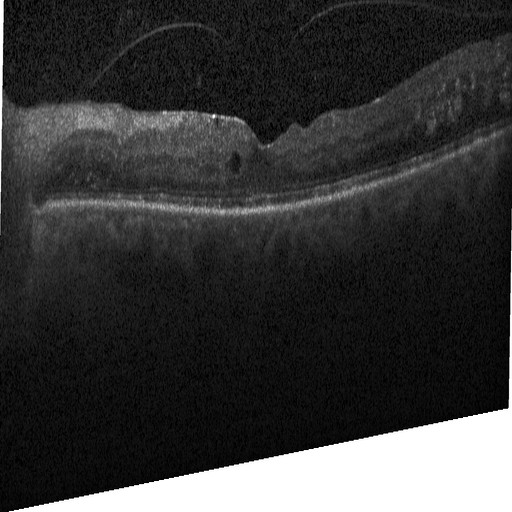 OCT scan showing diabetic macular edema.